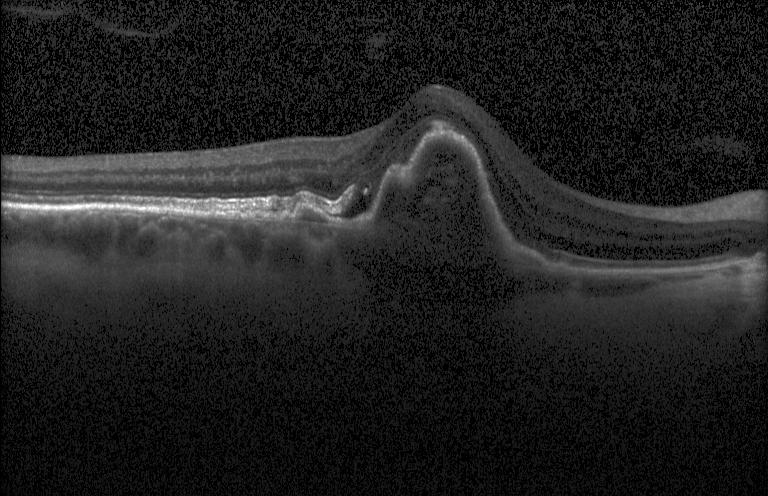

A choroidal neovascular membrane.